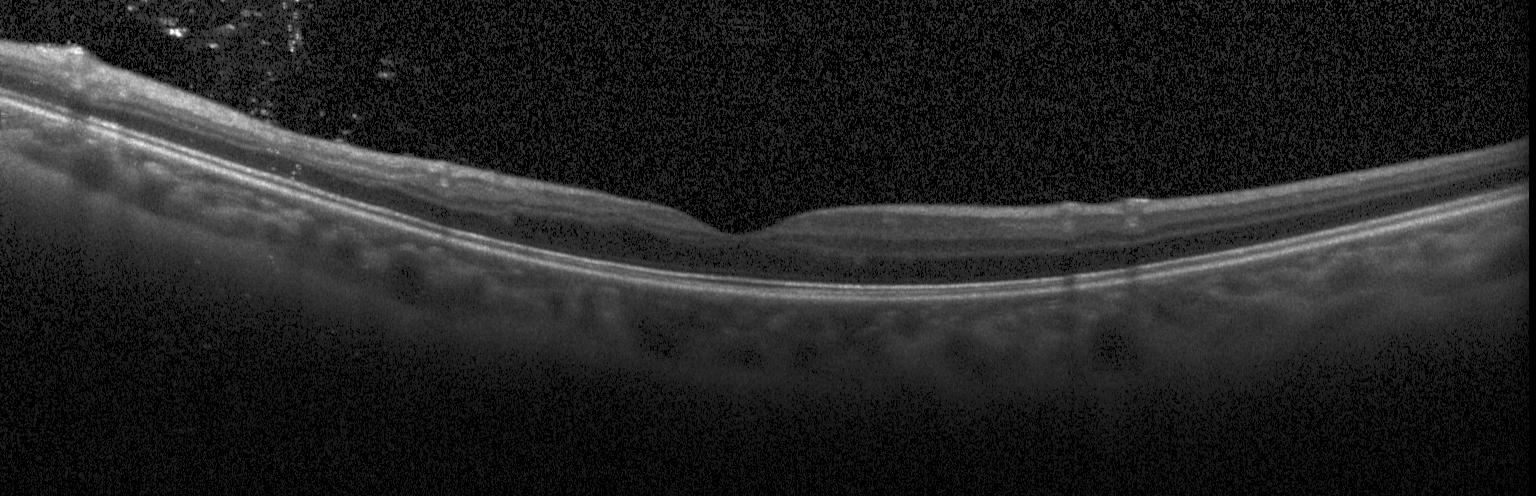

Assessment: no evidence of choroidal neovascularization, diabetic macular edema, or drusen.